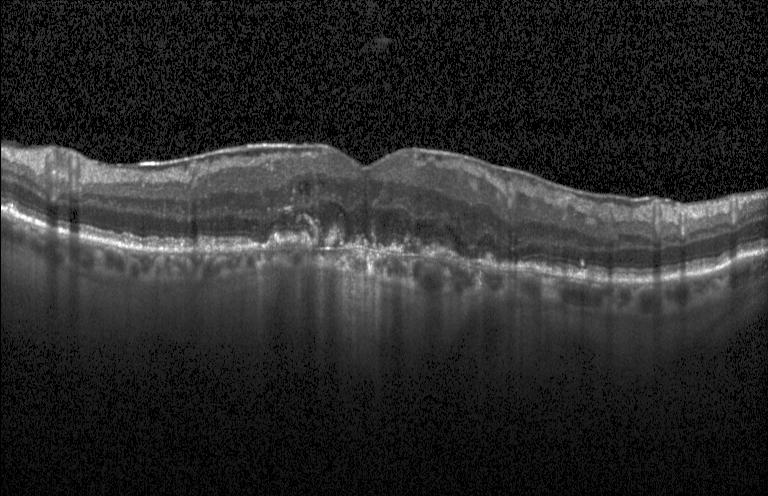

SD-OCT · horizontal scan through the fovea · retinal OCT B-scan · Heidelberg Spectralis OCT system
Impression: CNV.